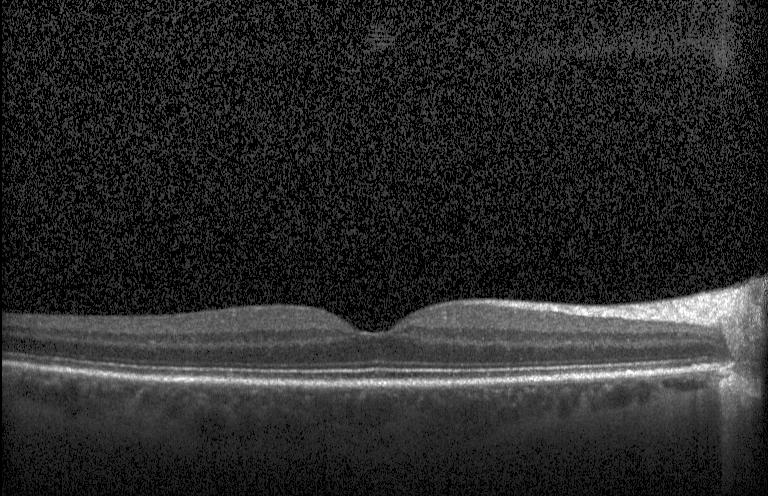 SD-OCT · horizontal scan through the fovea · OCT B-scan. The scan shows neither choroidal neovascularization, diabetic macular edema, nor drusen.